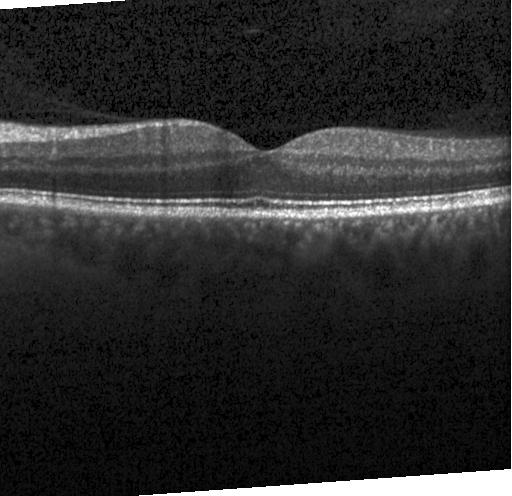 This B-scan demonstrates neither choroidal neovascularization, diabetic macular edema, nor drusen.